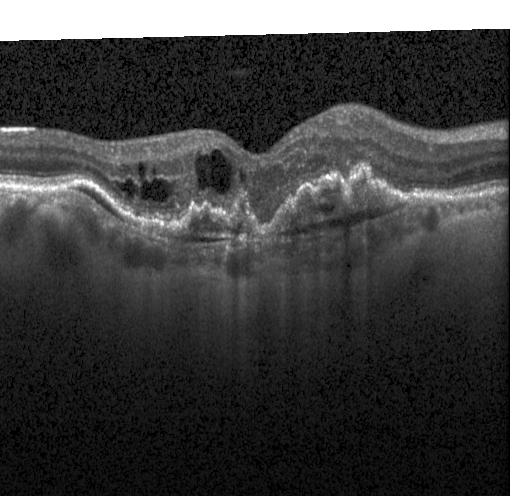

Through the macula · optical coherence tomography scan. Impression: a choroidal neovascular membrane.